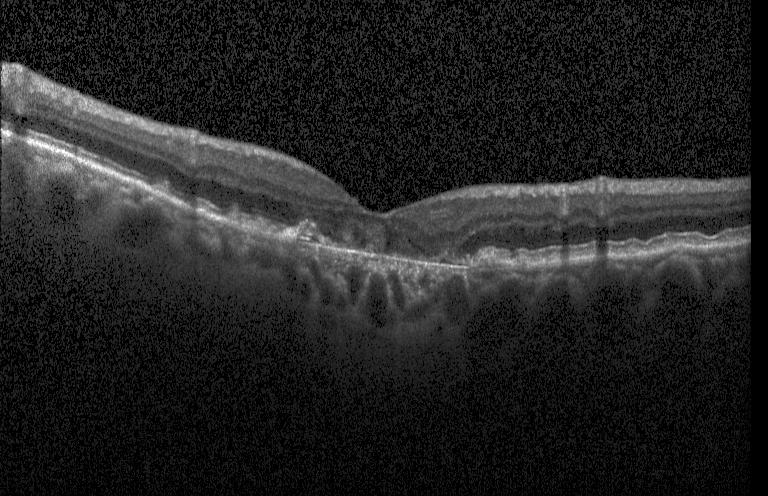

Diagnosis: choroidal neovascularization (CNV).